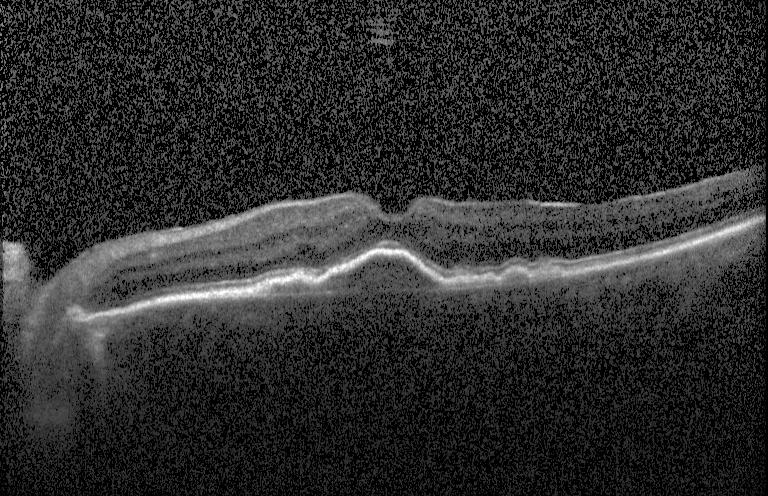 Retinal OCT cross-section. Heidelberg Spectralis OCT system. Spectral-domain optical coherence tomography. Finding: choroidal neovascularization (CNV).